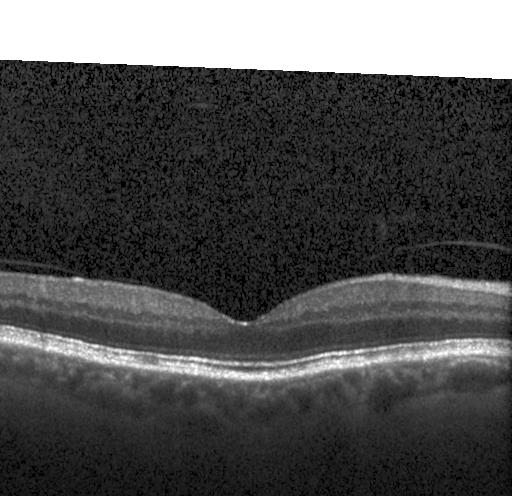

Macular OCT: no evidence of CNV, DME, or drusen.